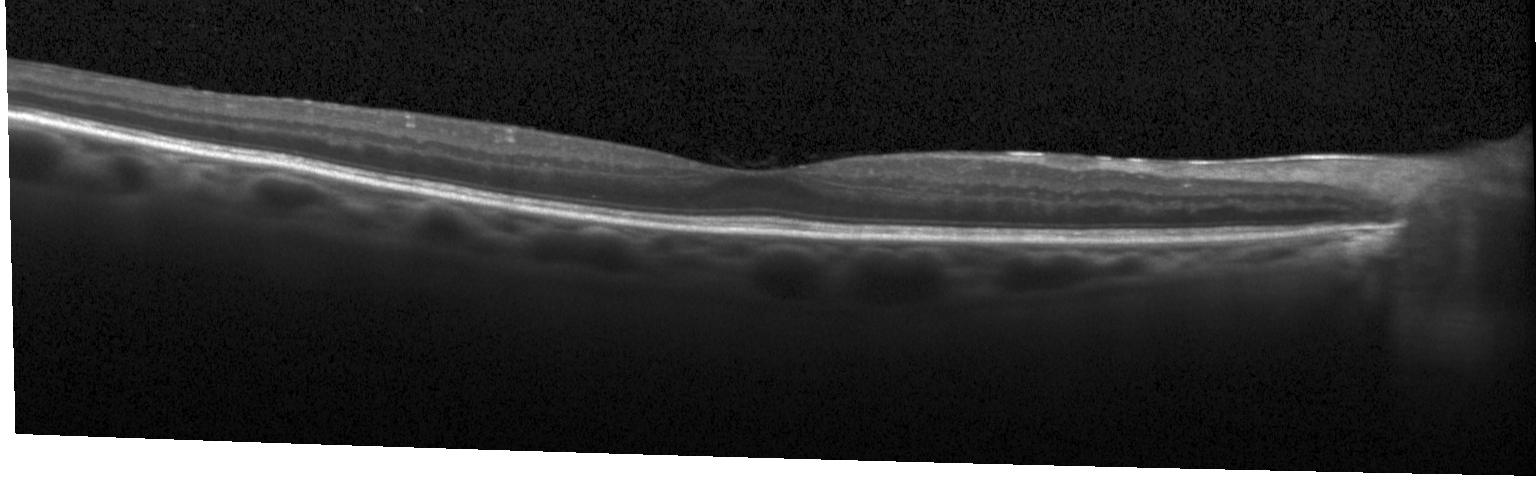
OCT line scan — Diagnosis: neither choroidal neovascularization, diabetic macular edema, nor drusen.